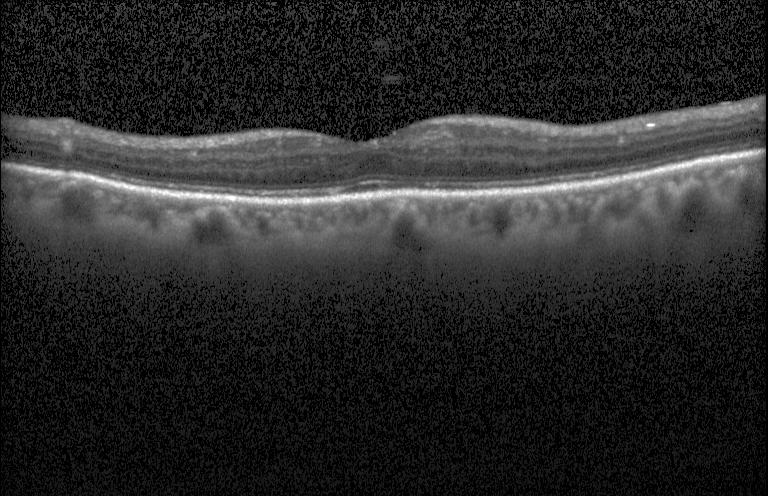 This B-scan demonstrates no evidence of CNV, DME, or drusen.